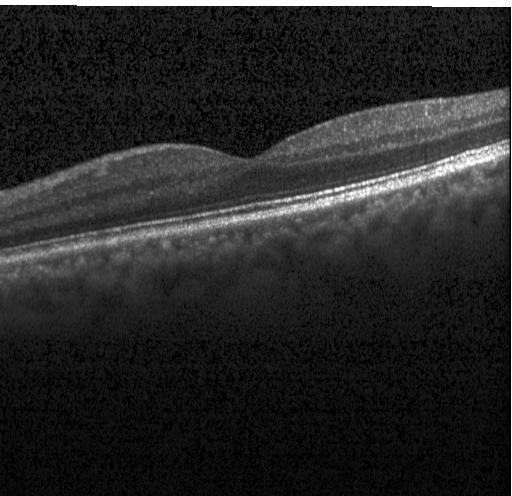

OCT line scan, acquired on a Heidelberg Spectralis. OCT finding: no CNV, DME, or drusen.